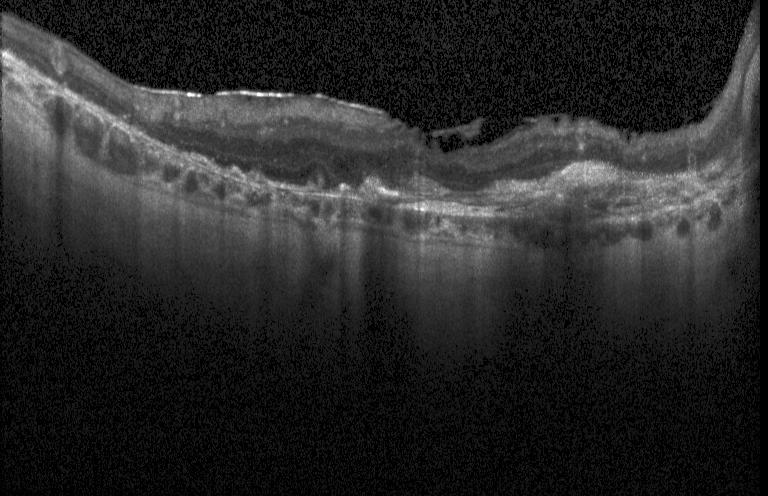

OCT finding: choroidal neovascularization (CNV).